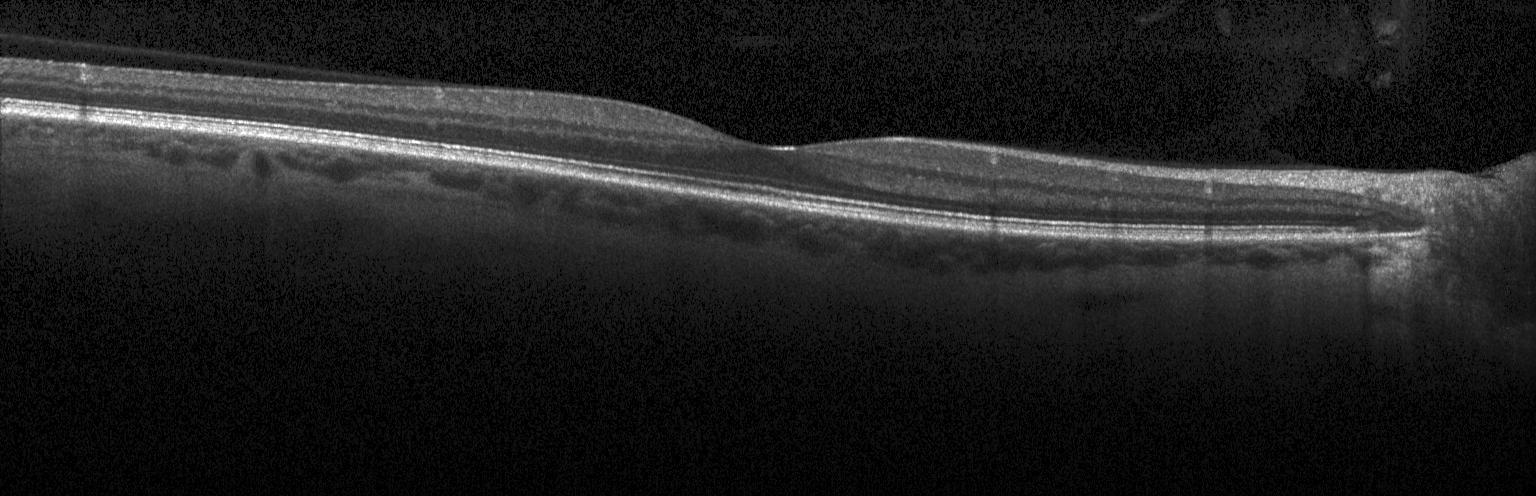

Retinal OCT cross-section, Heidelberg Spectralis, spectral-domain optical coherence tomography, macular scan
Diagnosis: no choroidal neovascularization, no diabetic macular edema, and no drusen.